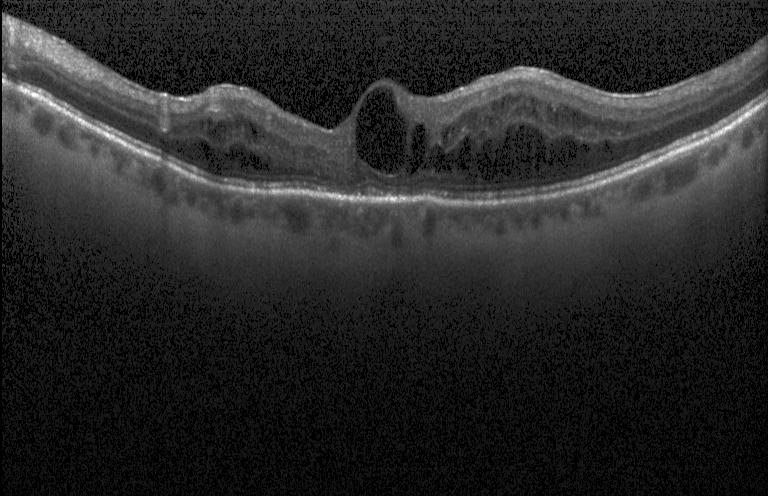
Retinal OCT cross-section, instrument: Heidelberg Spectralis, spectral-domain optical coherence tomography. Macular OCT: DME.